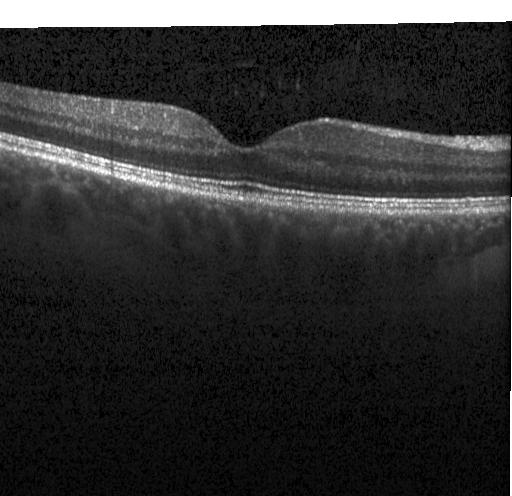
Instrument: Heidelberg Spectralis, OCT B-scan. Impression: no choroidal neovascularization, no diabetic macular edema, and no drusen.